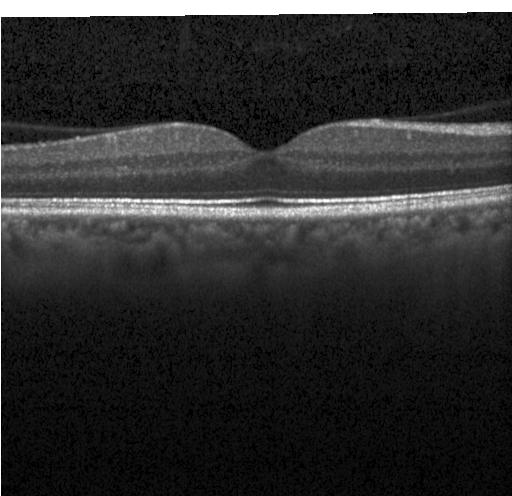

Diagnosis: no CNV, DME, or drusen.